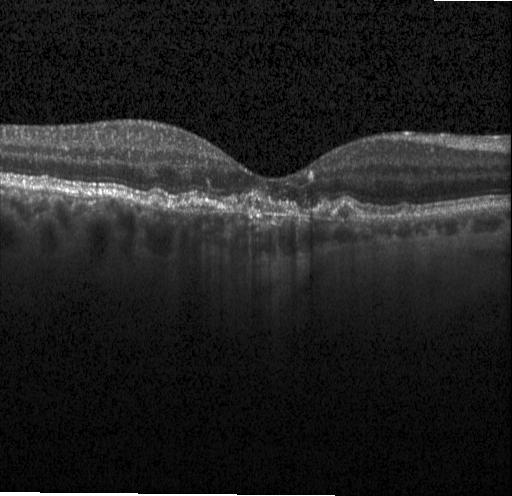 SD-OCT, OCT line scan, horizontal scan through the fovea, instrument: Heidelberg Spectralis. Finding: choroidal neovascularization.